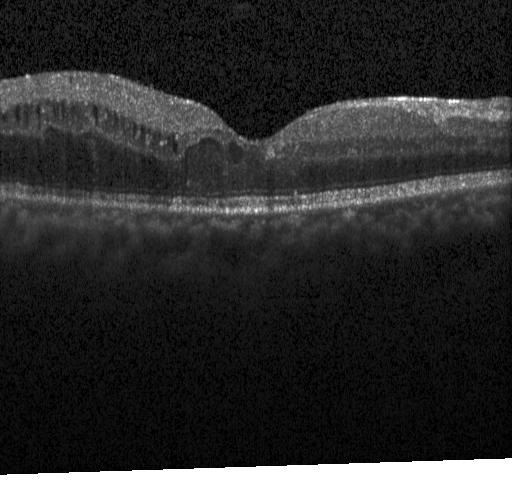

Optical coherence tomography scan. Fovea-centered.
OCT finding: DME.